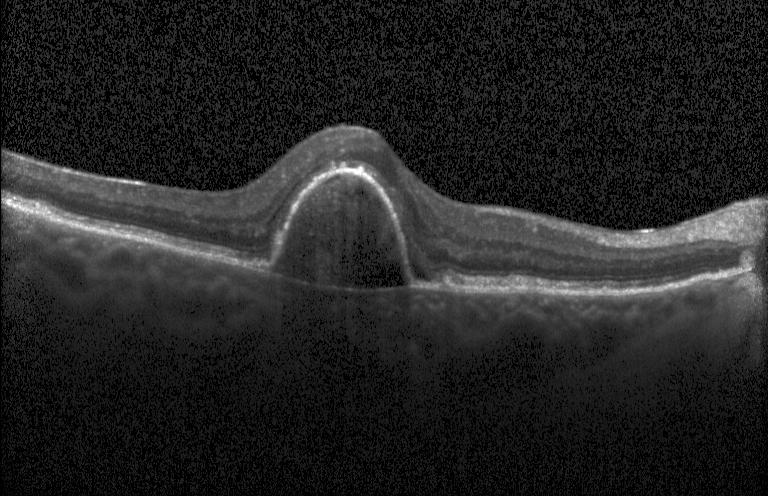
Heidelberg Spectralis OCT system, macular scan, spectral-domain optical coherence tomography, retinal OCT B-scan
Impression: CNV.